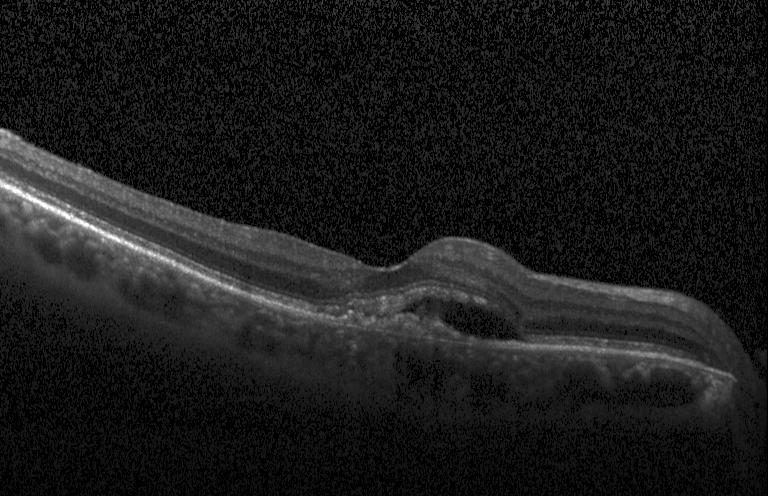

Optical coherence tomography scan, Heidelberg Spectralis OCT system — Impression: CNV.